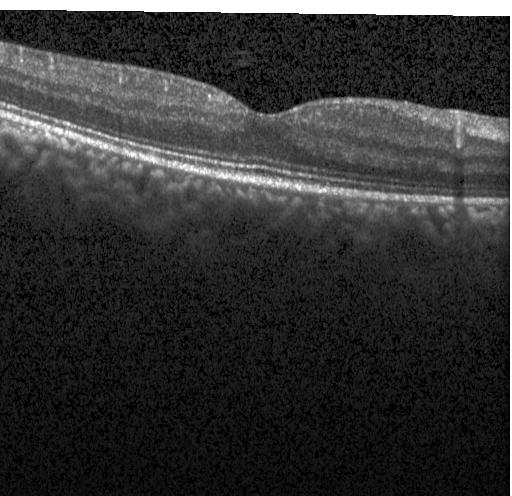 Impression: no choroidal neovascularization, diabetic macular edema, or drusen.